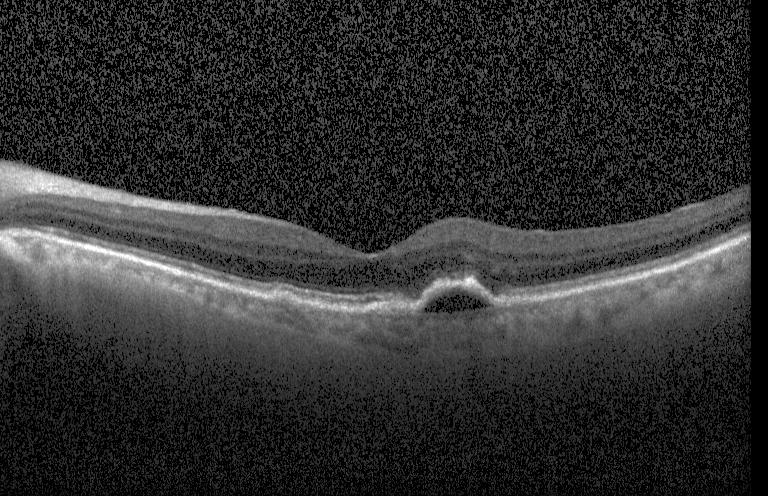

OCT finding: choroidal neovascularization.